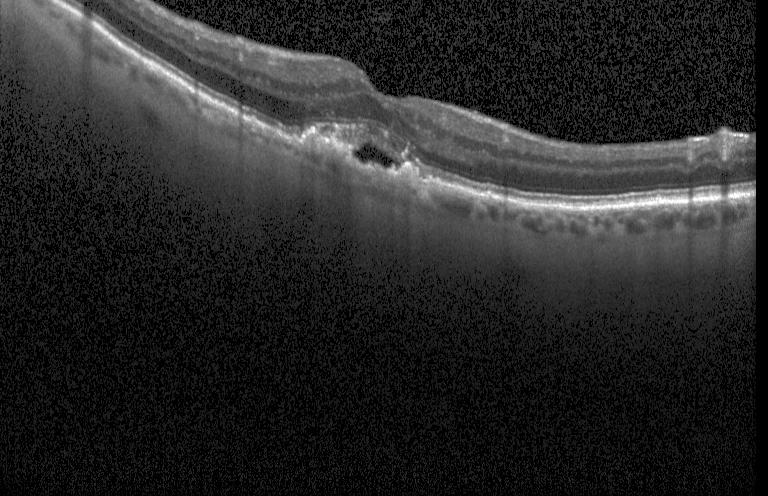

This B-scan demonstrates choroidal neovascularization.